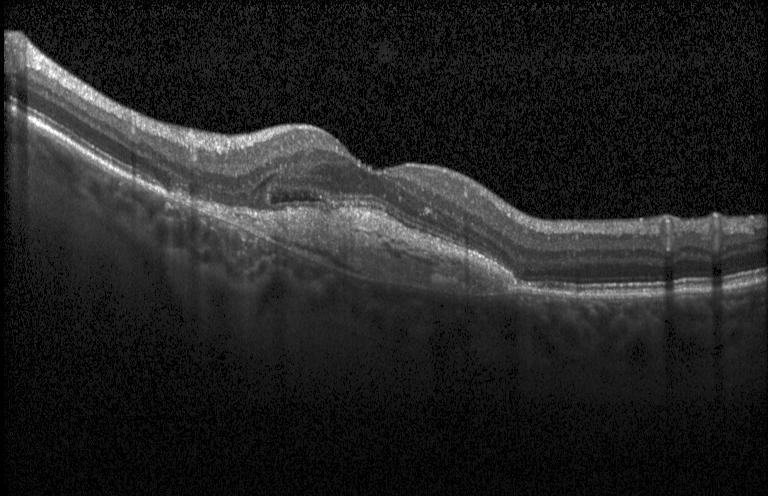 Instrument: Heidelberg Spectralis. Spectral-domain OCT. Optical coherence tomography B-scan. Fovea-centered.
This B-scan demonstrates choroidal neovascularization.